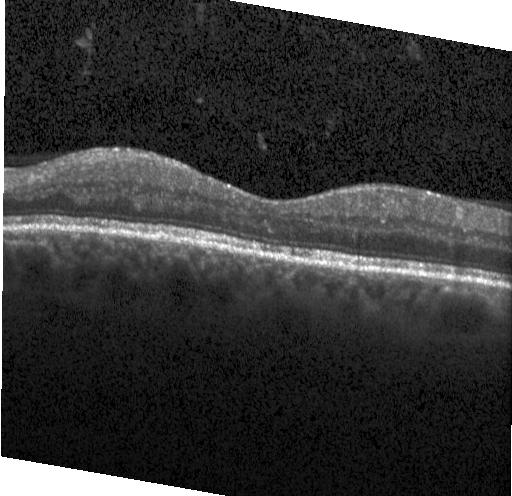
The scan shows no CNV, no DME, and no drusen.